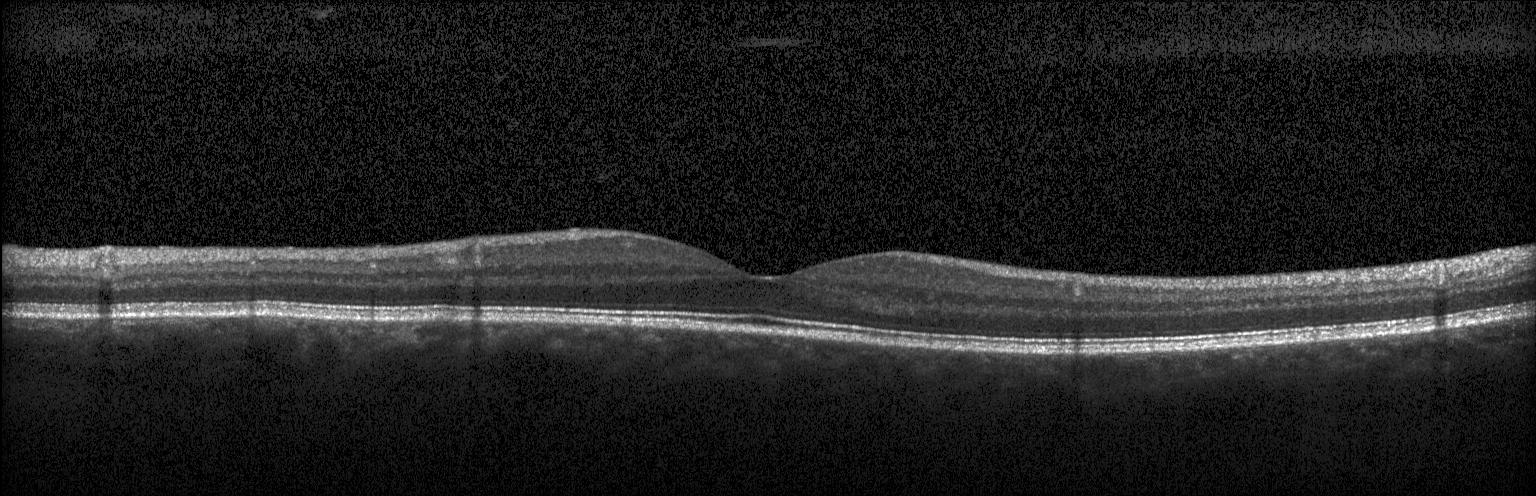

Instrument: Heidelberg Spectralis. Retinal OCT cross-section. SD-OCT.
This B-scan demonstrates no CNV, no DME, and no drusen.